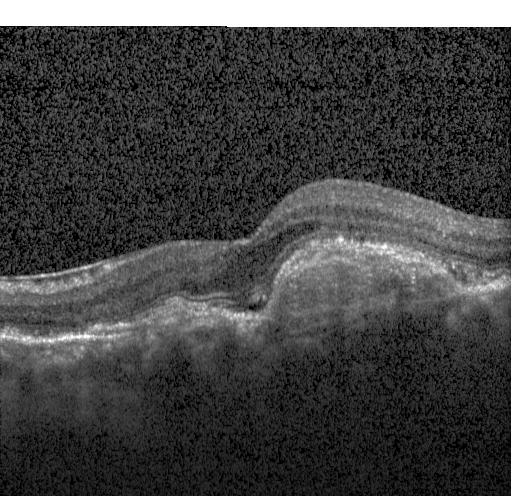

Macular OCT: CNV.